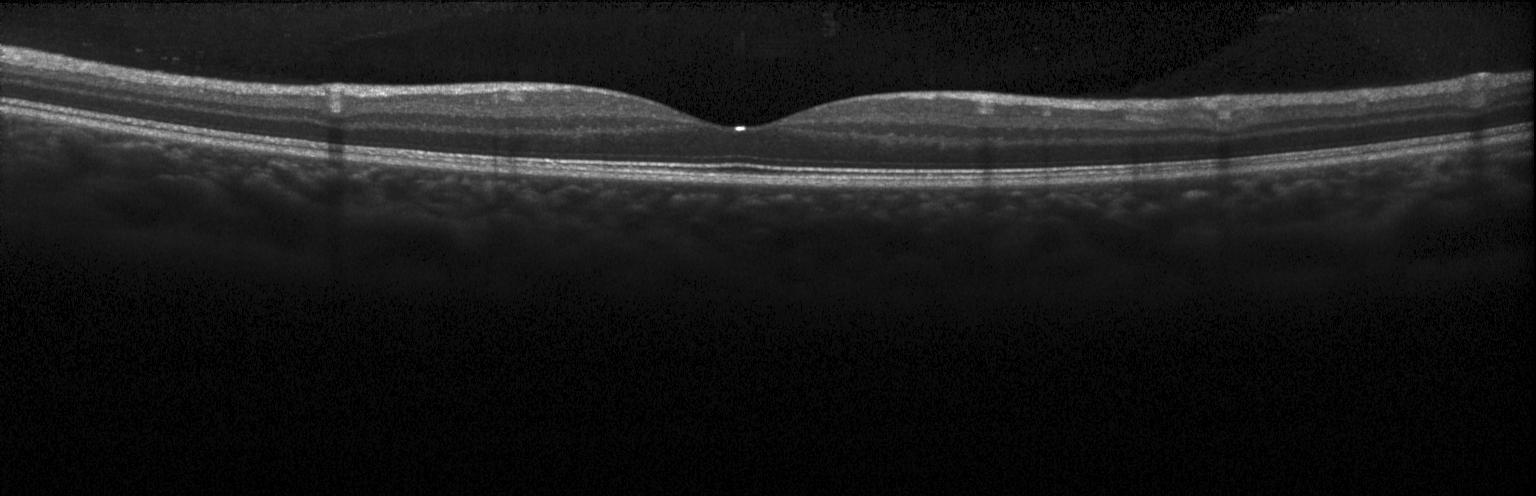
This B-scan demonstrates no choroidal neovascularization, diabetic macular edema, or drusen.